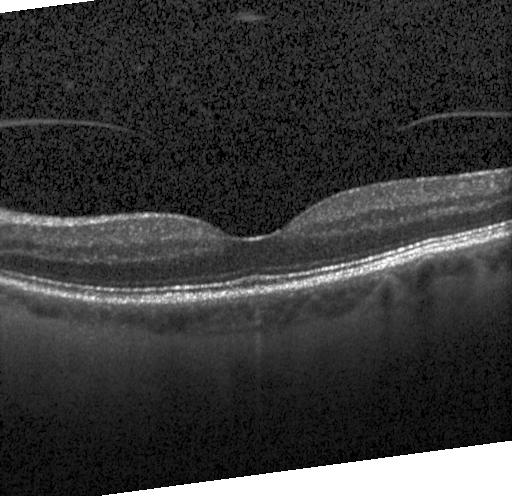

Optical coherence tomography B-scan
This B-scan demonstrates no choroidal neovascularization, no diabetic macular edema, and no drusen.